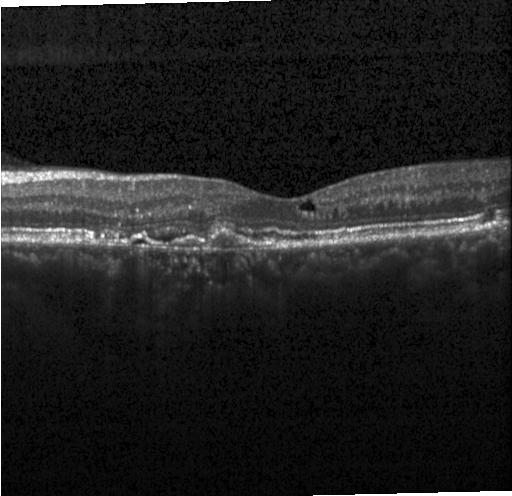 Optical coherence tomography B-scan; SD-OCT
Finding: a choroidal neovascular membrane.